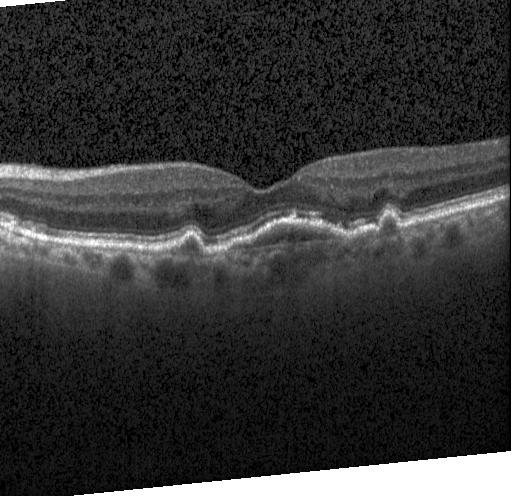

Dx: choroidal neovascularization (CNV).